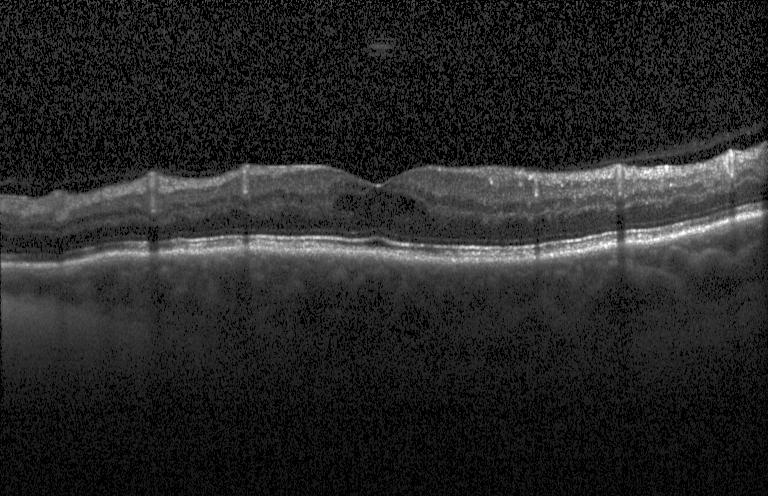
OCT finding: diabetic macular edema (DME).